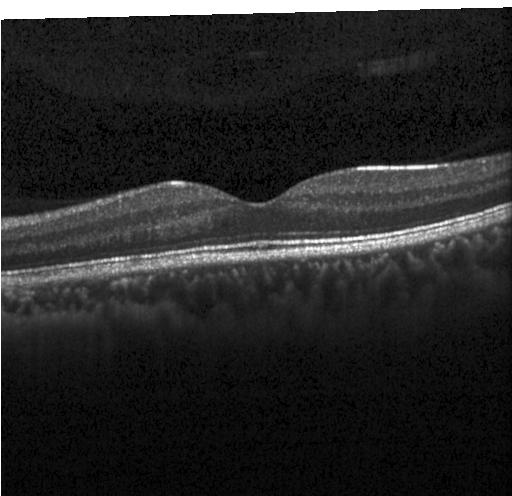

Optical coherence tomography scan. Spectral-domain OCT. Heidelberg Spectralis.
Dx: neither CNV, DME, nor drusen.